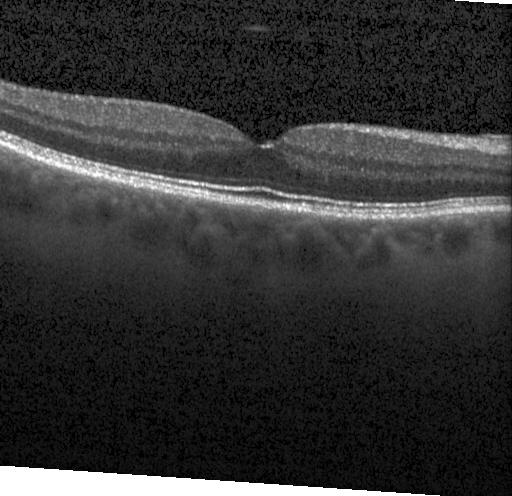 No CNV, no DME, and no drusen.